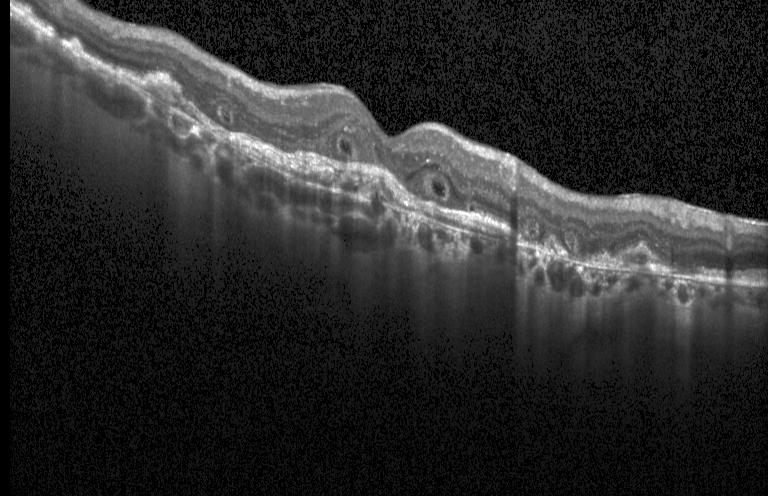
OCT finding: CNV.